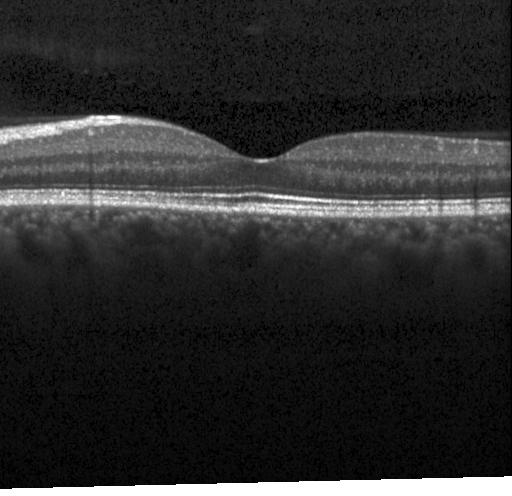
Assessment: neither CNV, DME, nor drusen.